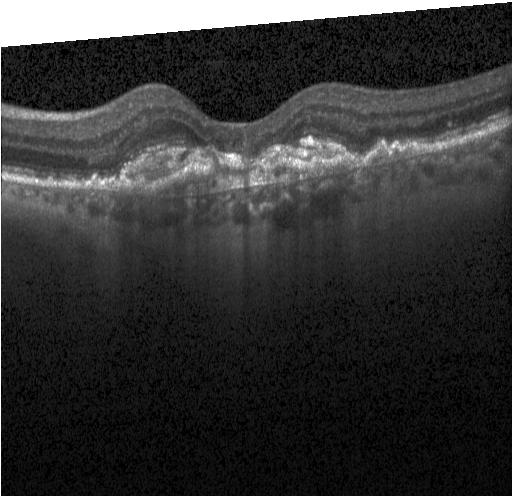 OCT B-scan.
Impression: a choroidal neovascular membrane.